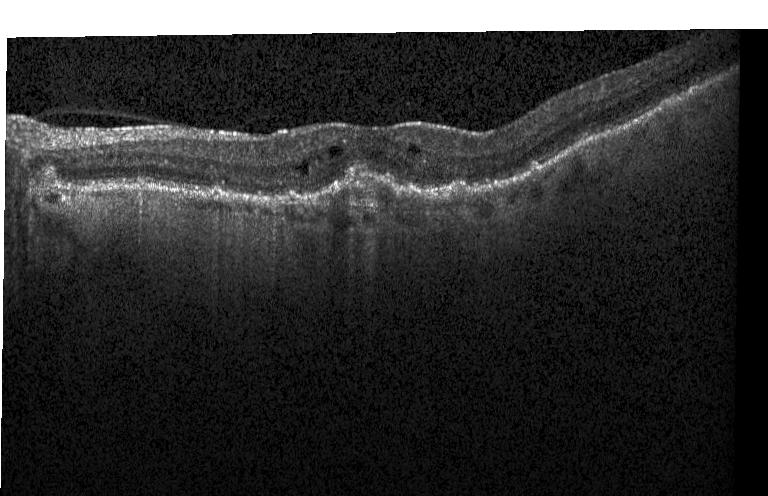
Retinal OCT B-scan.
Macular OCT: choroidal neovascularization (CNV).